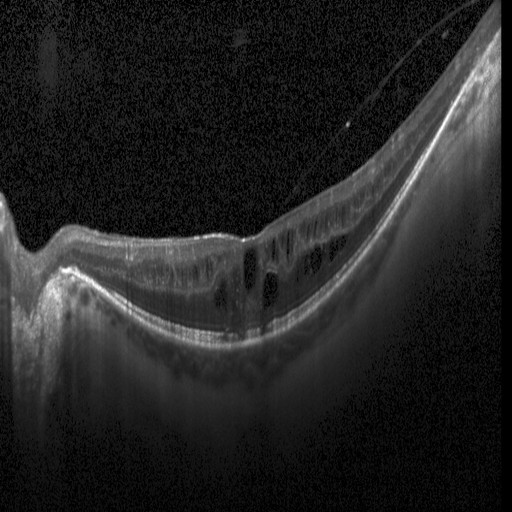
Diagnosis: diabetic macular edema.